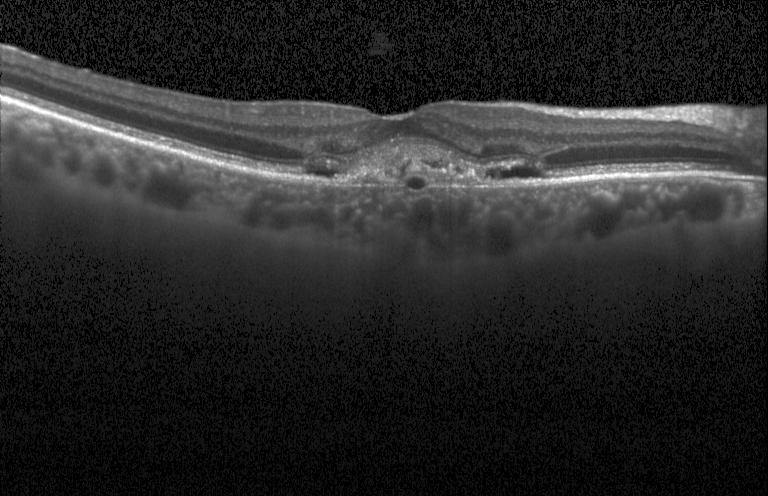
Optical coherence tomography B-scan. This B-scan demonstrates a choroidal neovascular membrane.